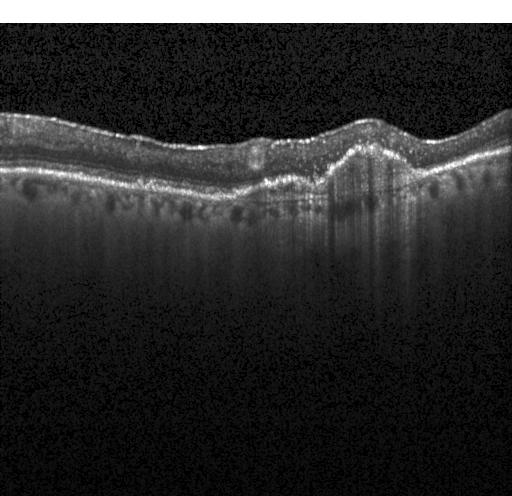 Through the macula; acquired on a Heidelberg Spectralis; optical coherence tomography B-scan; spectral-domain OCT — A choroidal neovascular membrane.